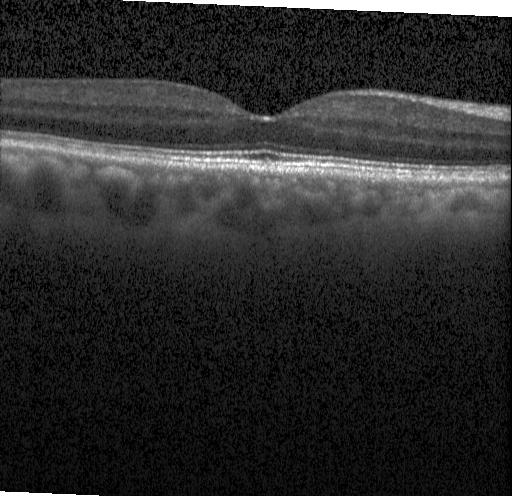

Diagnosis: no evidence of CNV, DME, or drusen.